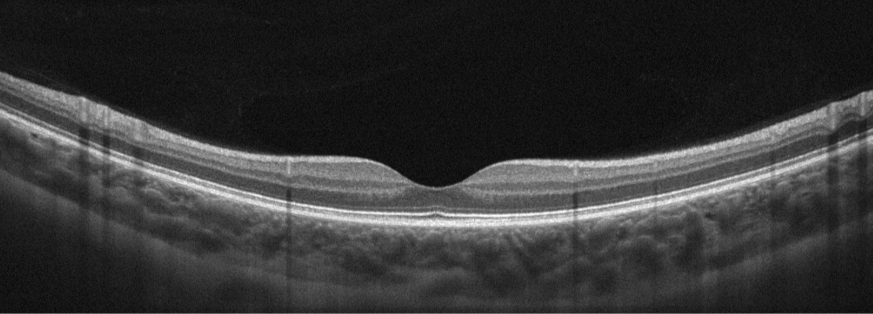
Optical coherence tomography scan. Acquired on an Optovue Avanti RTVue XR. Macular scan.
Diagnosis: no AMD, DME, ERM, RAO, RVO, or VID.